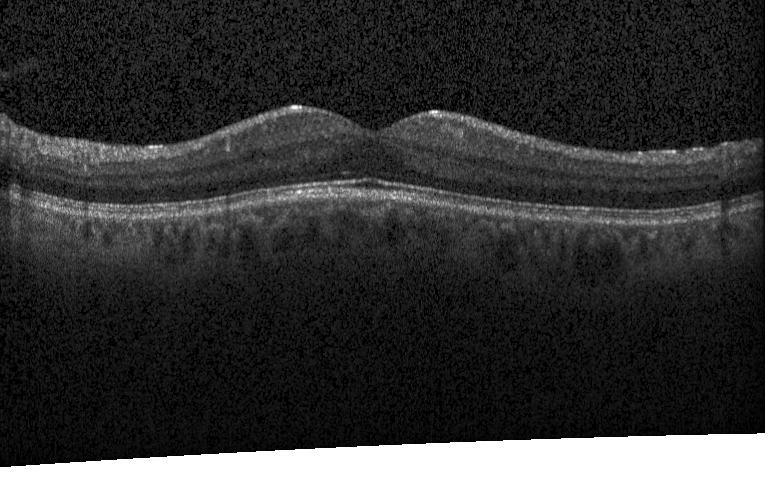
Finding: neither CNV, DME, nor drusen.